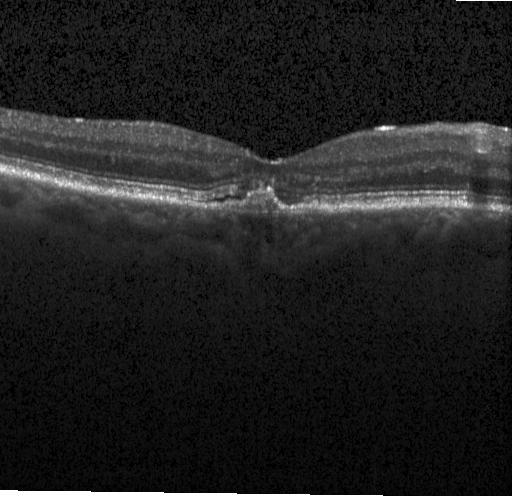 Macular OCT: choroidal neovascularization (CNV).